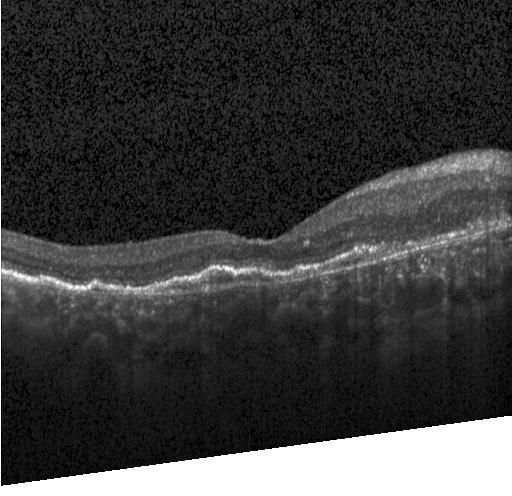 Optical coherence tomography scan · Heidelberg Spectralis OCT system · fovea-centered.
Impression: CNV.